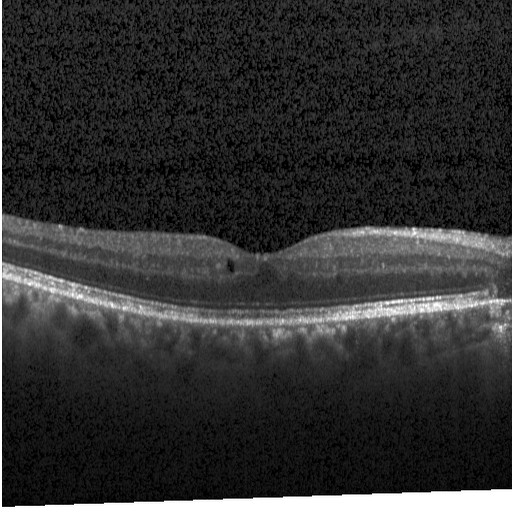

Assessment: DME.